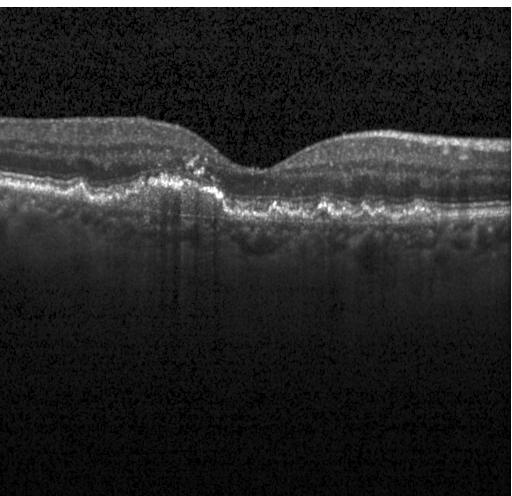 Optical coherence tomography scan. The scan shows a choroidal neovascular membrane.